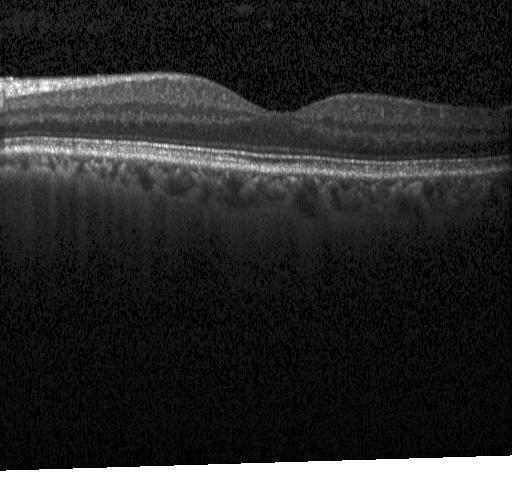
Impression: no choroidal neovascularization, no diabetic macular edema, and no drusen.